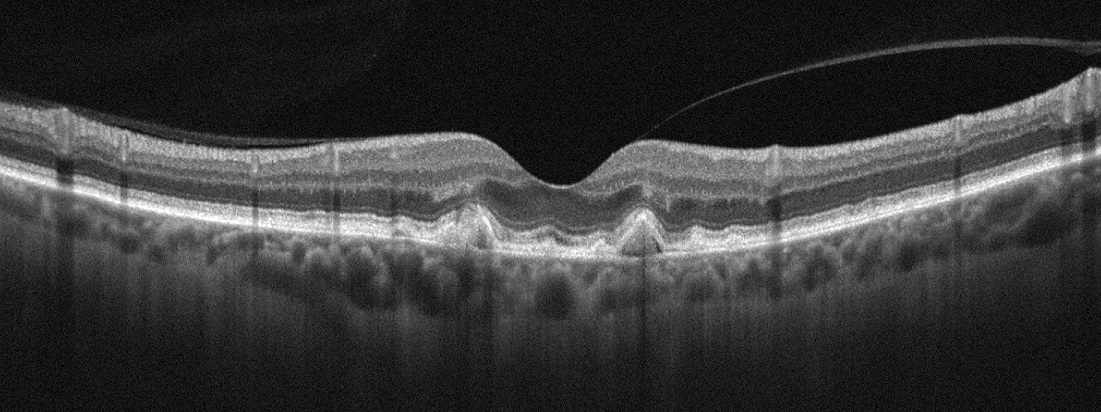
Macular OCT: age-related macular degeneration.